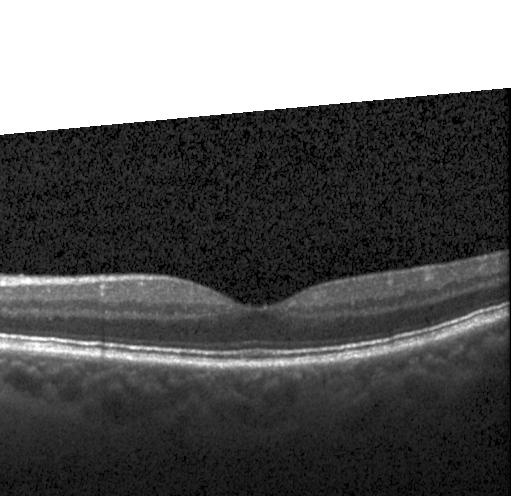
OCT B-scan. This B-scan demonstrates no CNV, DME, or drusen.